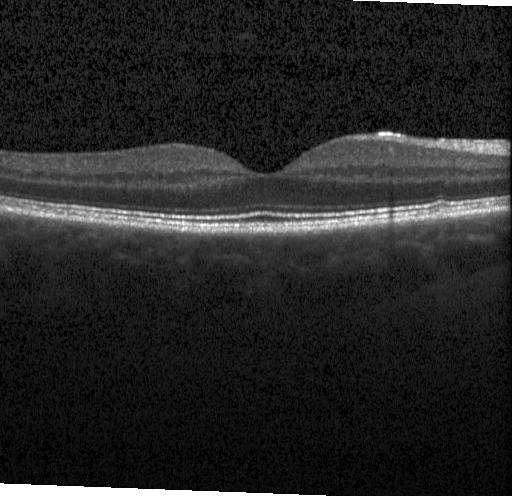

Optical coherence tomography scan. Instrument: Heidelberg Spectralis. Horizontal scan through the fovea. The scan shows no choroidal neovascularization, no diabetic macular edema, and no drusen.